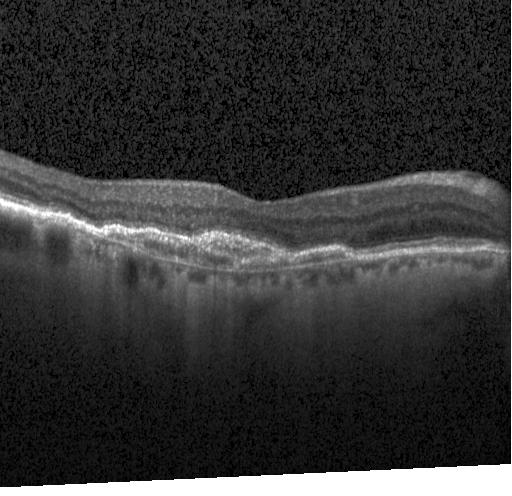 Centered on the fovea, optical coherence tomography scan. The scan shows choroidal neovascularization.